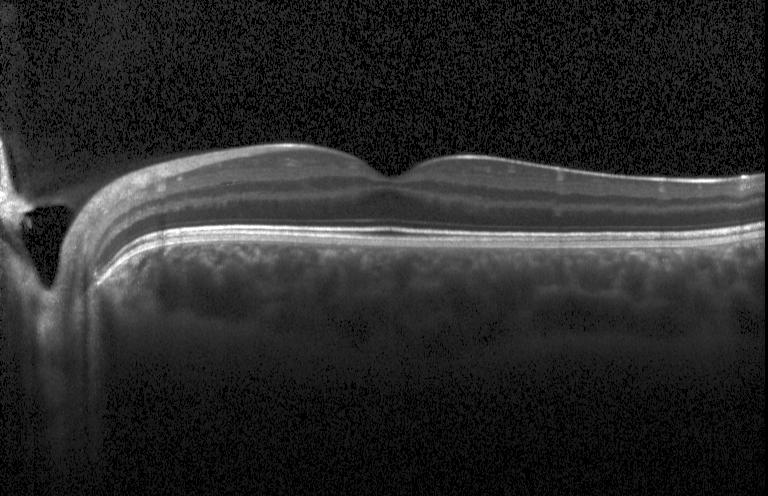
Optical coherence tomography scan · centered on the fovea.
This B-scan demonstrates no evidence of choroidal neovascularization, diabetic macular edema, or drusen.